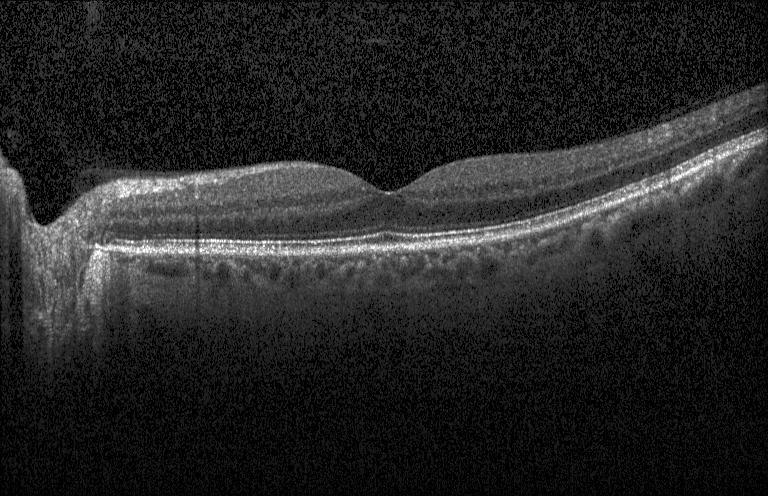
Retinal OCT cross-section; Heidelberg Spectralis OCT system.
Impression: no evidence of choroidal neovascularization, diabetic macular edema, or drusen.